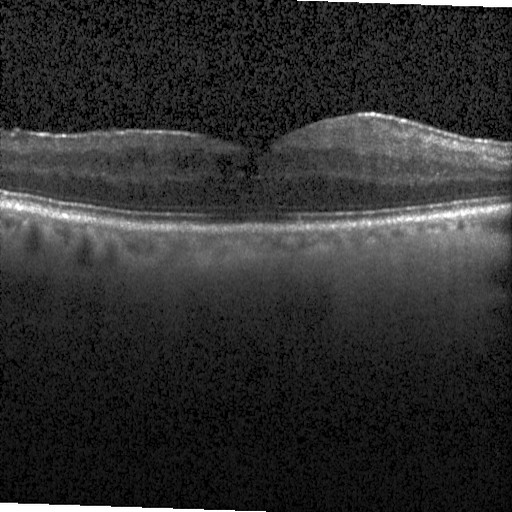 Optical coherence tomography B-scan, horizontal scan through the fovea, spectral-domain optical coherence tomography.
Diagnosis: diabetic macular edema (DME).